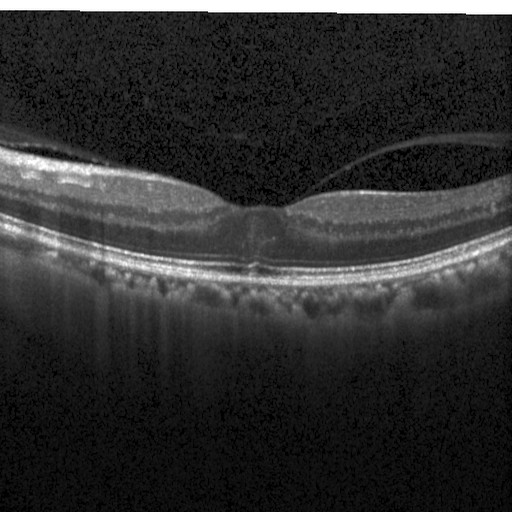

Centered on the fovea. Spectral-domain OCT. Instrument: Heidelberg Spectralis. OCT B-scan. Dx: DME.